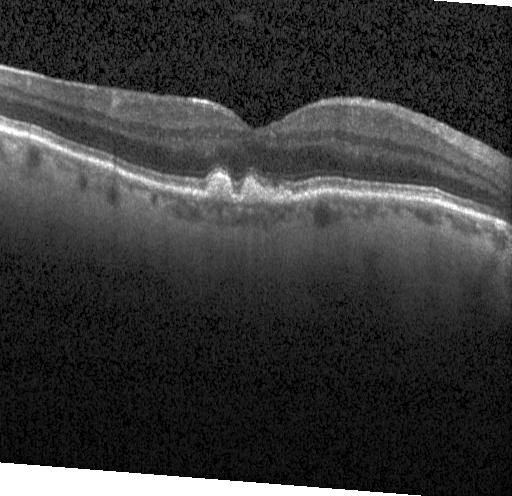

Impression: drusen.